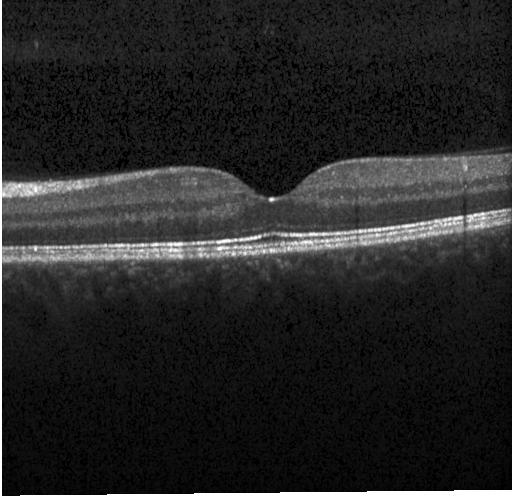 OCT line scan. Heidelberg Spectralis. Spectral-domain optical coherence tomography
The scan shows no choroidal neovascularization, no diabetic macular edema, and no drusen.